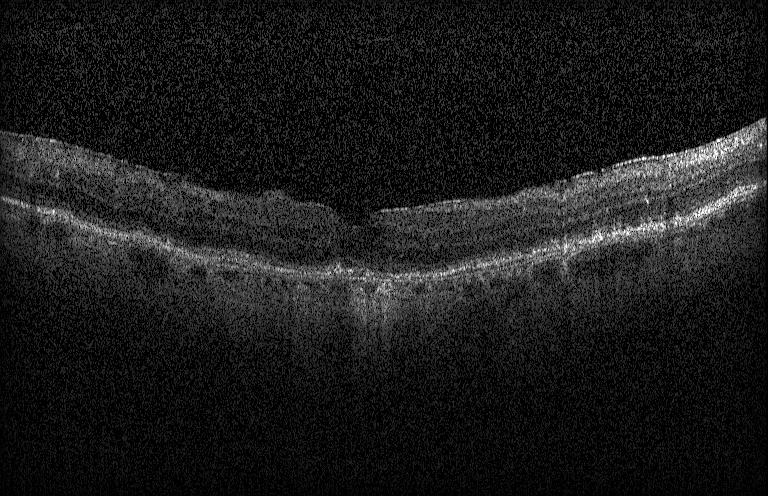 Acquired on a Heidelberg Spectralis. Fovea-centered. OCT B-scan. Assessment: no choroidal neovascularization, diabetic macular edema, or drusen.